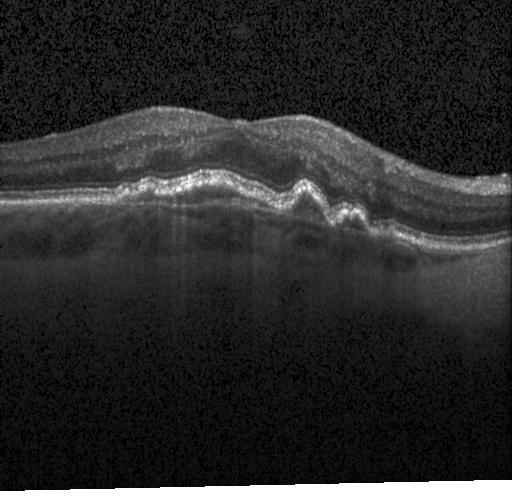

Optical coherence tomography B-scan; Heidelberg Spectralis.
Dx: choroidal neovascularization.